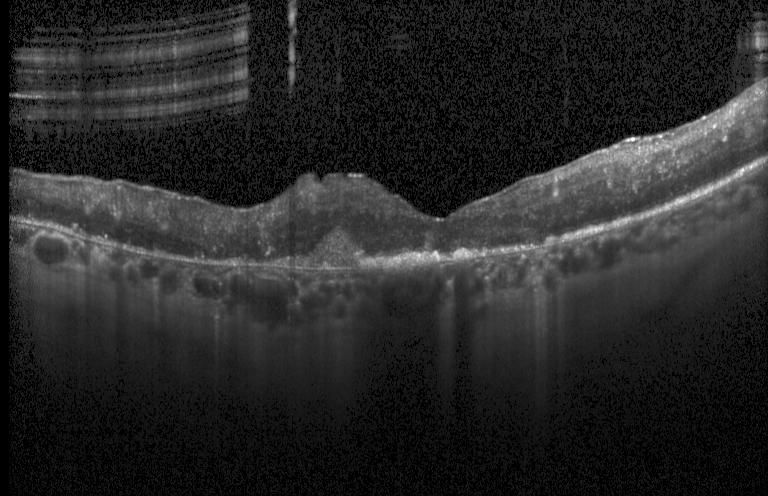

Finding: choroidal neovascularization.